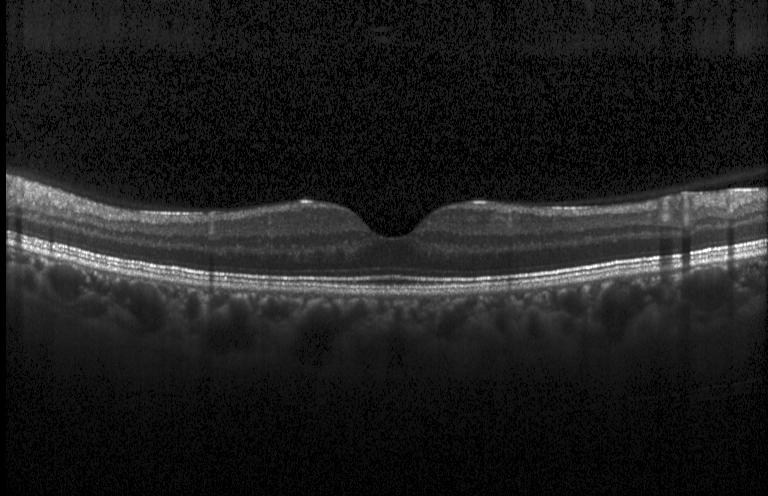 Retinal OCT cross-section — This B-scan demonstrates no choroidal neovascularization, diabetic macular edema, or drusen.